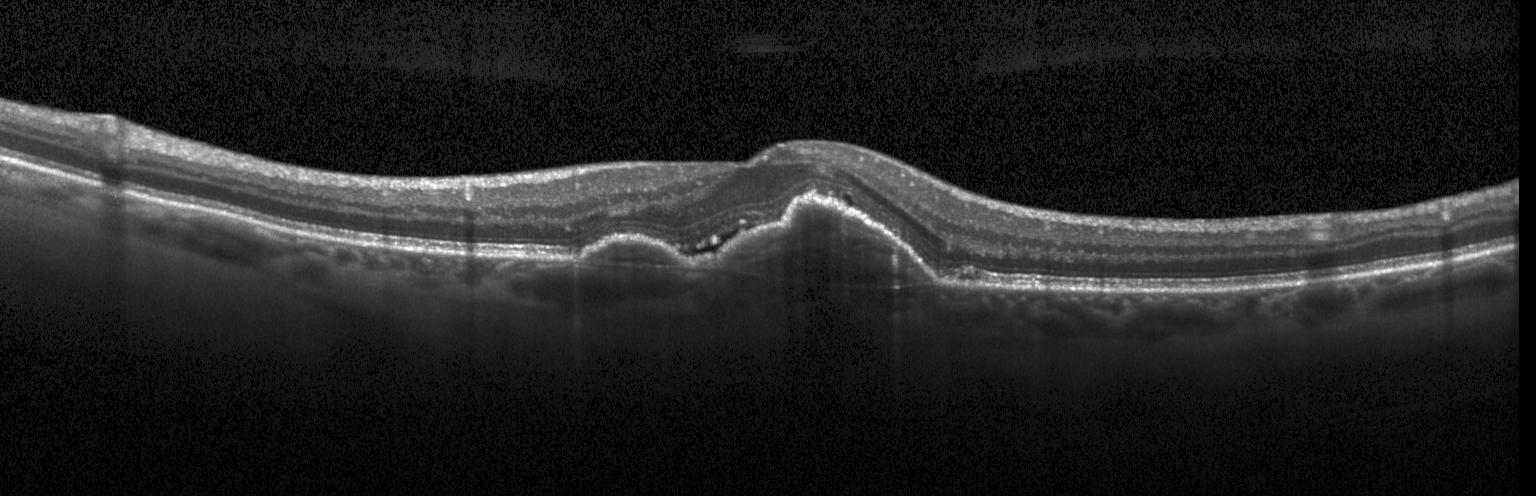 Optical coherence tomography B-scan. Macular scan
Impression: a choroidal neovascular membrane.